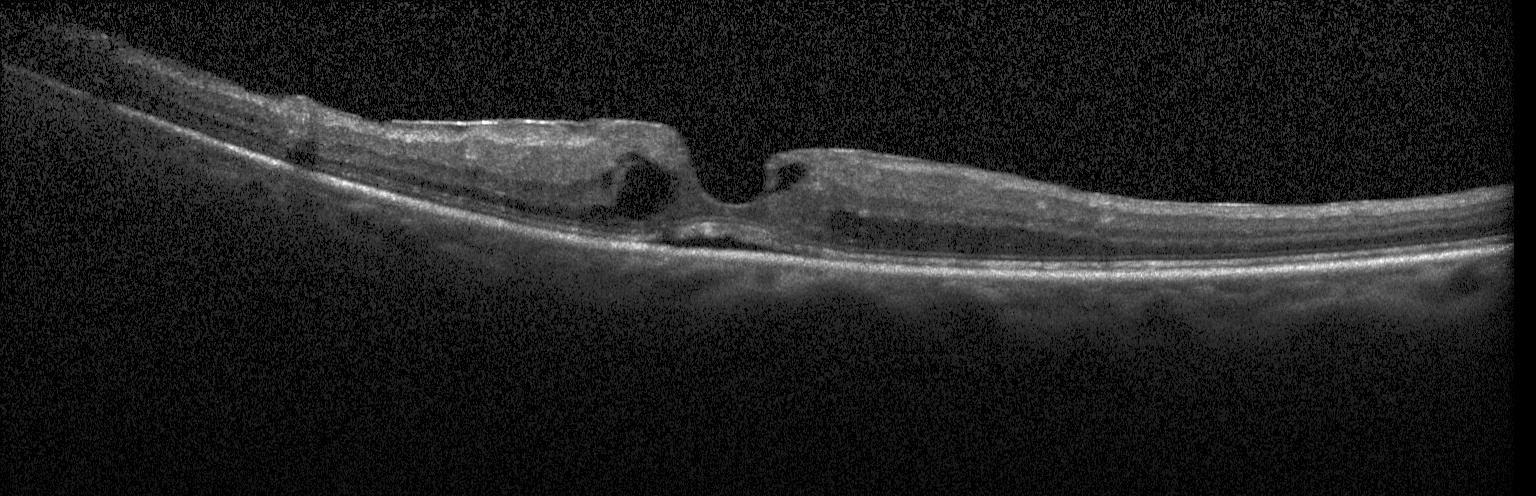
OCT B-scan showing diabetic macular edema (DME).